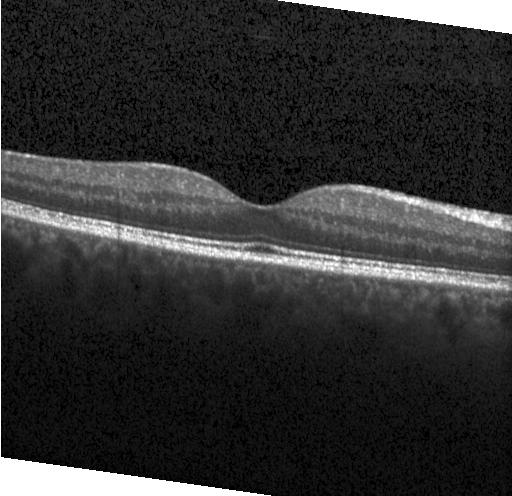

Retinal OCT B-scan; horizontal scan through the fovea. Finding: no choroidal neovascularization, diabetic macular edema, or drusen.